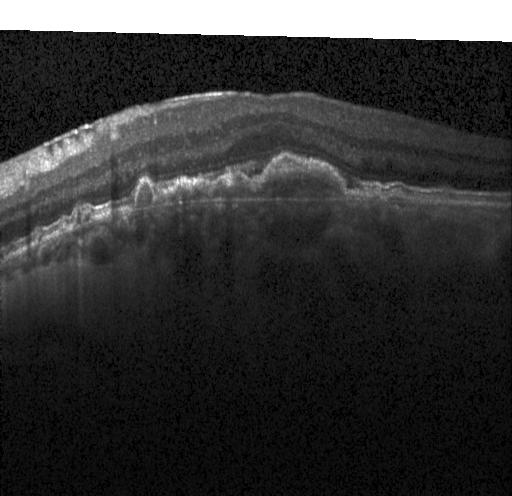
SD-OCT, retinal OCT B-scan
Macular OCT: a choroidal neovascular membrane.